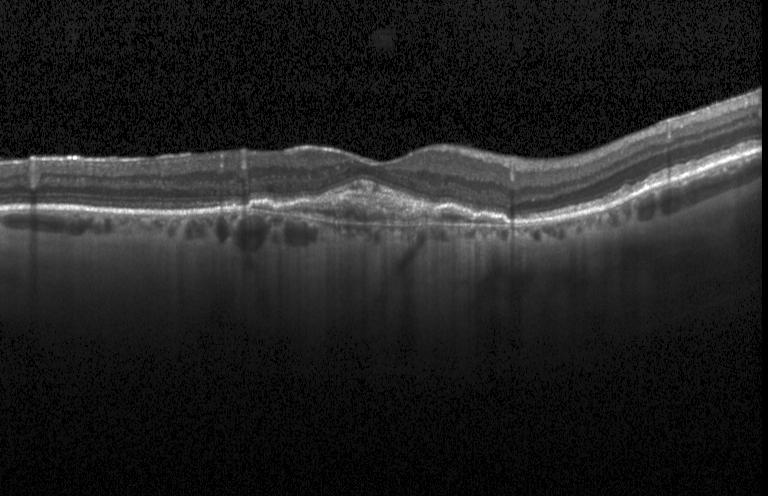 Optical coherence tomography scan; Heidelberg Spectralis OCT system; macular scan; spectral-domain optical coherence tomography
Finding: choroidal neovascularization.